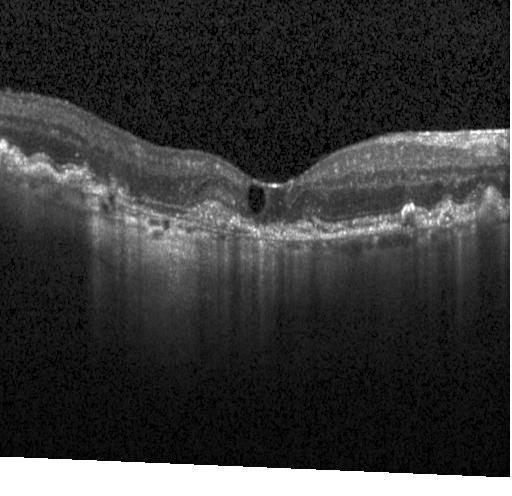 OCT finding: choroidal neovascularization (CNV).